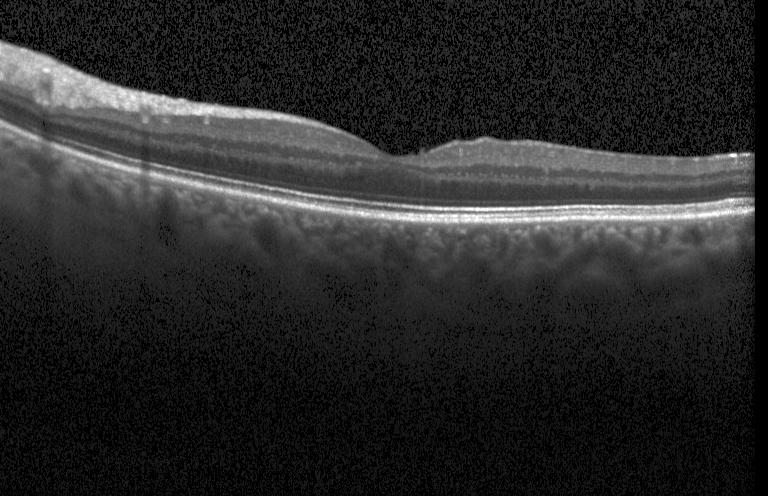

Heidelberg Spectralis; fovea-centered; retinal OCT B-scan. This B-scan demonstrates no evidence of choroidal neovascularization, diabetic macular edema, or drusen.